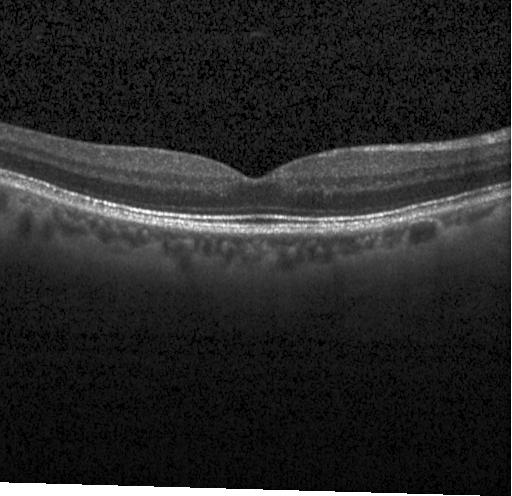 Diagnosis: no CNV, no DME, and no drusen.